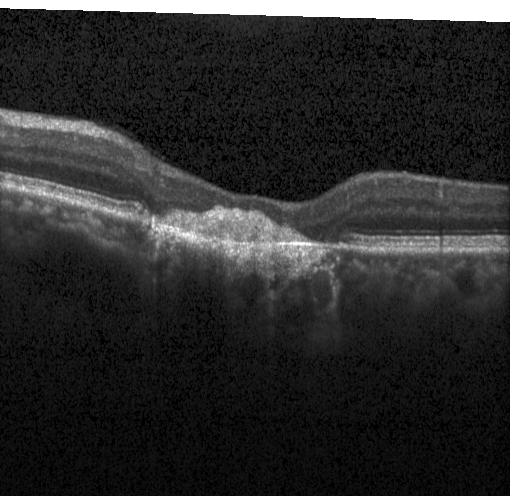
Heidelberg Spectralis OCT system. Retinal OCT cross-section. This B-scan demonstrates CNV.